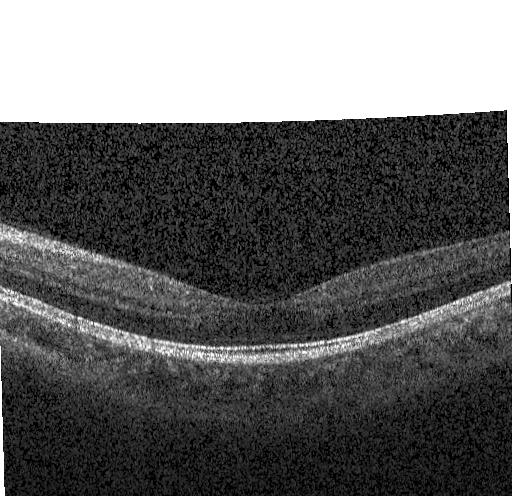

Finding: no choroidal neovascularization, no diabetic macular edema, and no drusen.